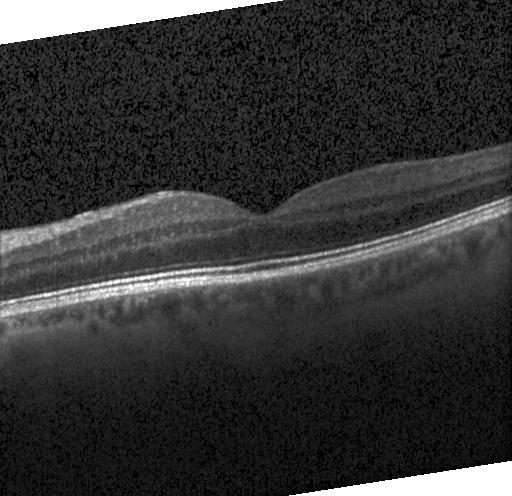
Instrument: Heidelberg Spectralis. Spectral-domain optical coherence tomography. Optical coherence tomography scan
Diagnosis: no choroidal neovascularization, diabetic macular edema, or drusen.